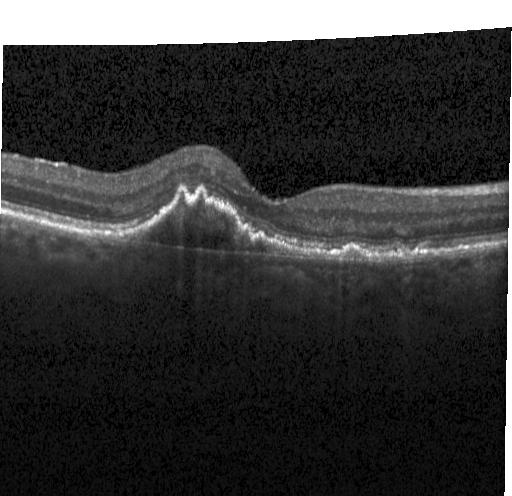 Impression: choroidal neovascularization.